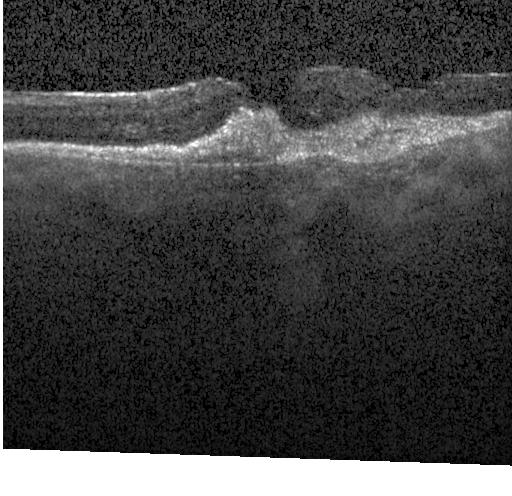 Spectral-domain optical coherence tomography · acquired on a Heidelberg Spectralis · OCT B-scan — The scan shows a choroidal neovascular membrane.